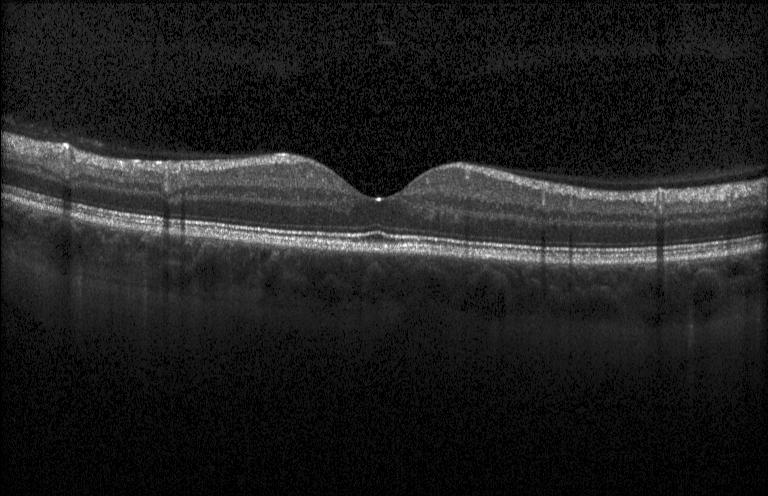 OCT line scan, instrument: Heidelberg Spectralis, through the macula. This B-scan demonstrates no choroidal neovascularization, diabetic macular edema, or drusen.